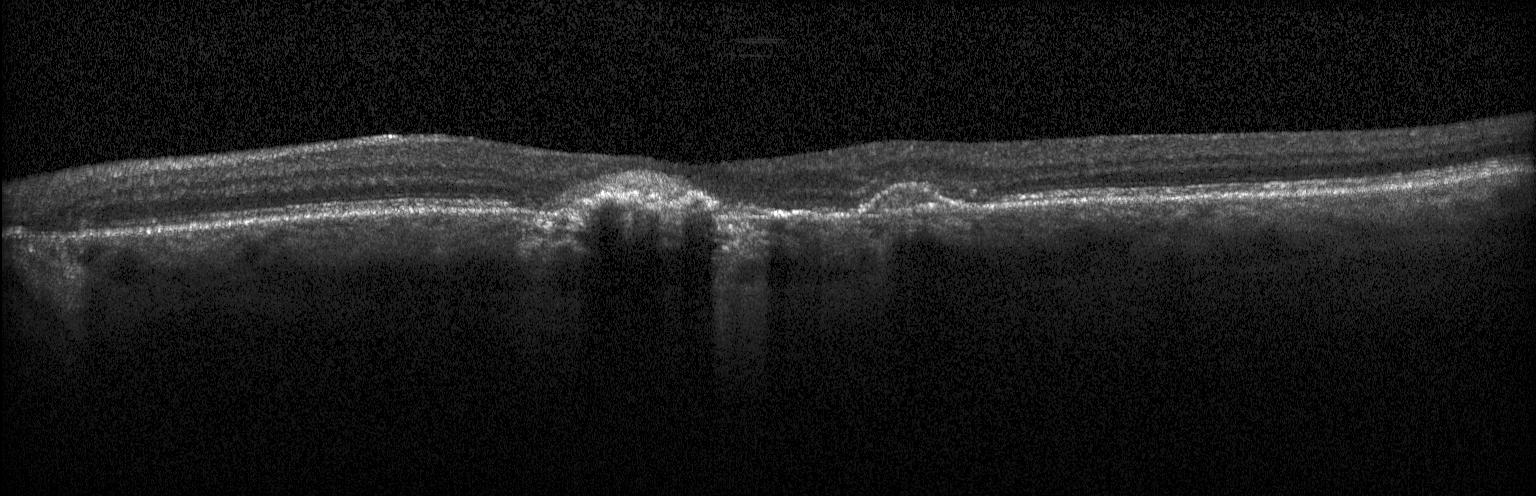
Choroidal neovascularization.